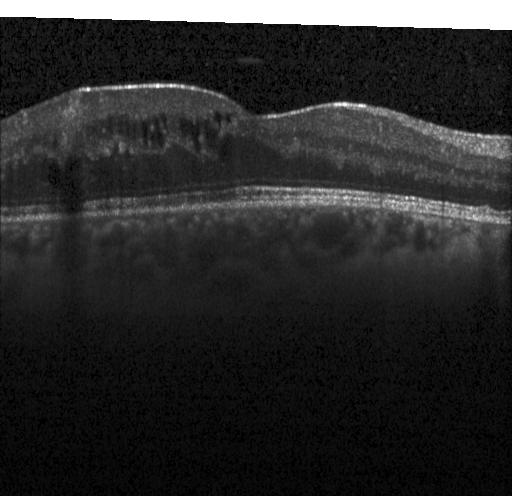

The scan shows diabetic macular edema.